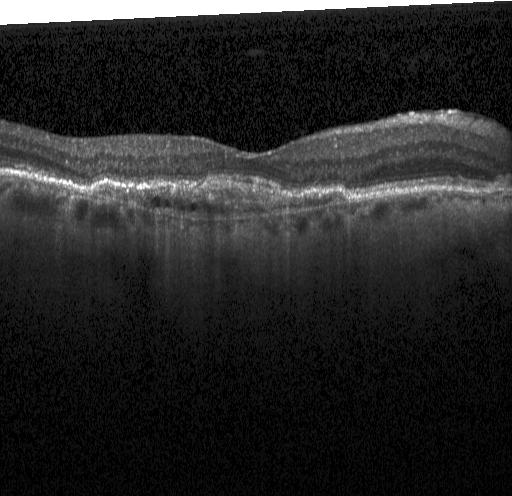
Instrument: Heidelberg Spectralis. Optical coherence tomography scan. Fovea-centered.
Diagnosis: choroidal neovascularization (CNV).